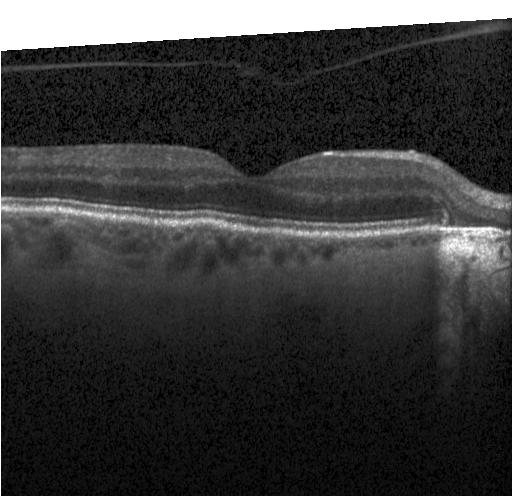
Through the macula · retinal OCT cross-section · Heidelberg Spectralis
Impression: no CNV, no DME, and no drusen.